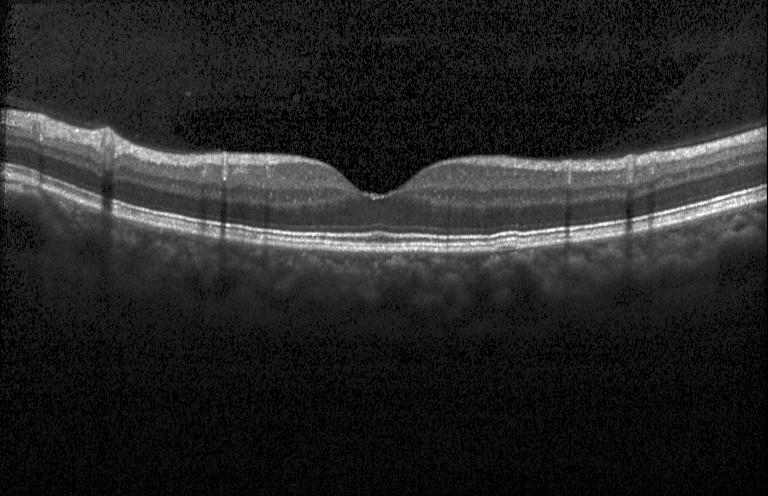 Through the macula; retinal OCT cross-section. OCT finding: no evidence of choroidal neovascularization, diabetic macular edema, or drusen.